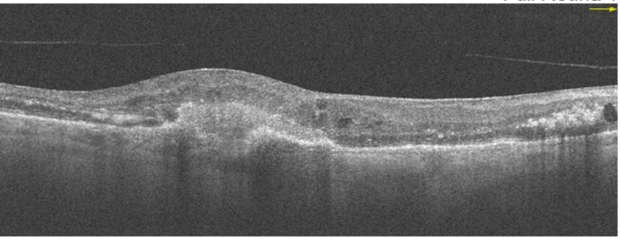

OCT B-scan
The scan shows age-related macular degeneration.